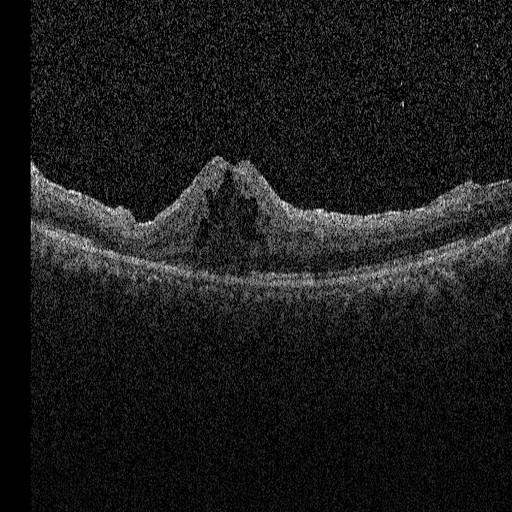
Diagnosis: diabetic macular edema (DME).